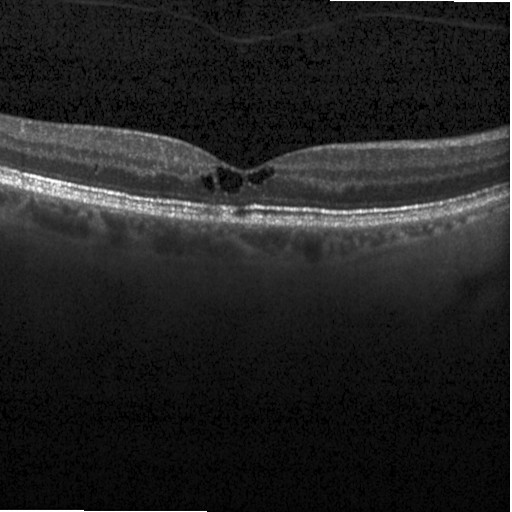 Spectral-domain OCT B-scan: DME.